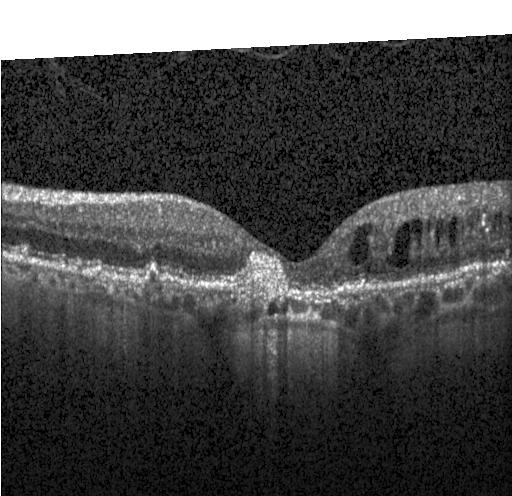
Retinal OCT cross-section · macular scan.
The scan shows choroidal neovascularization.